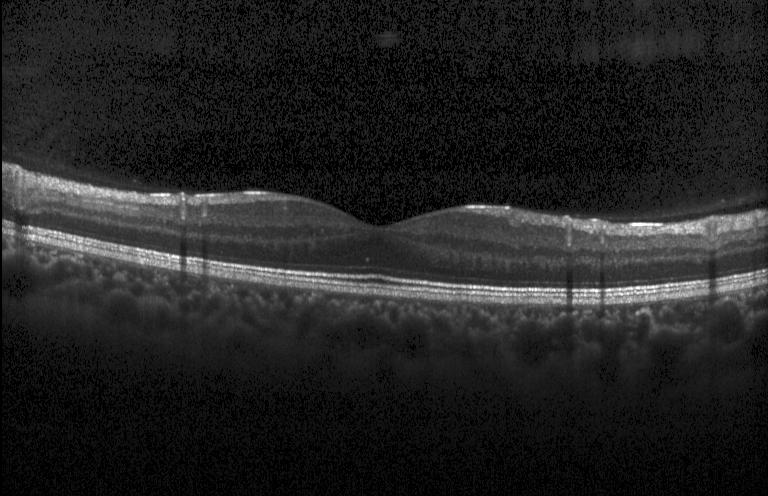

Spectral-domain OCT, Heidelberg Spectralis OCT system, fovea-centered, retinal OCT cross-section
This B-scan demonstrates neither choroidal neovascularization, diabetic macular edema, nor drusen.